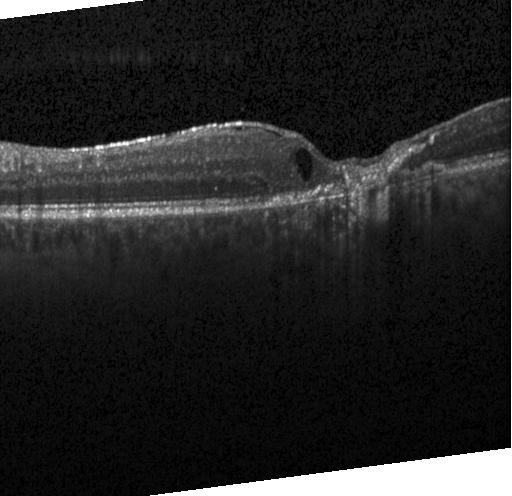
Finding: CNV.